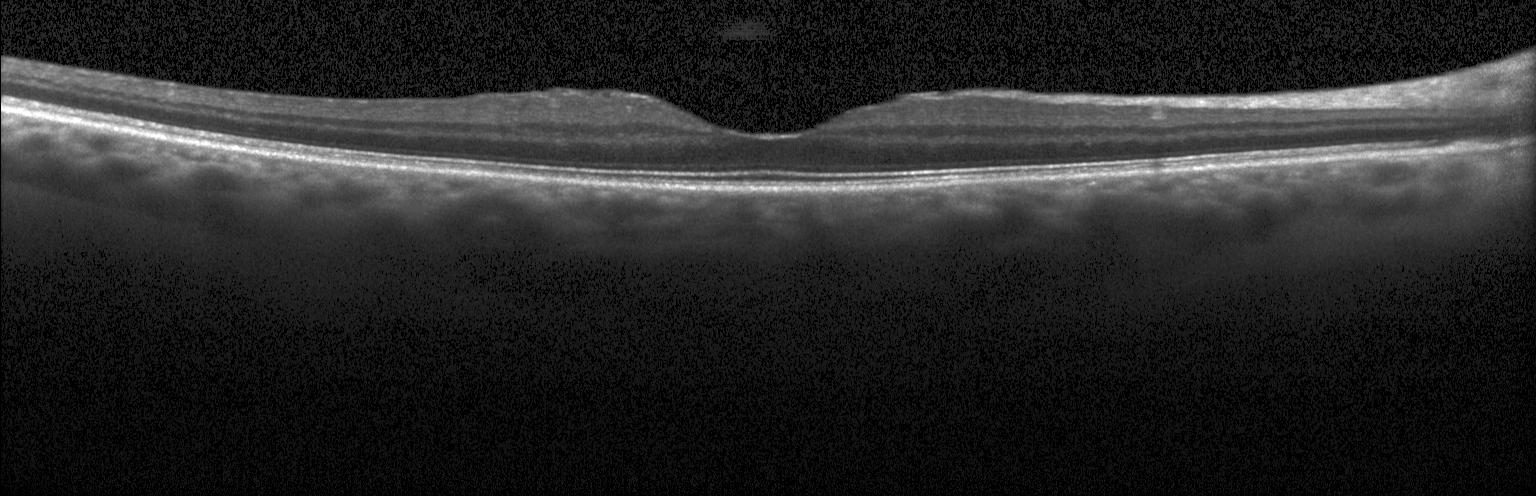

Spectral-domain OCT, fovea-centered, OCT line scan. Macular OCT: no CNV, DME, or drusen.